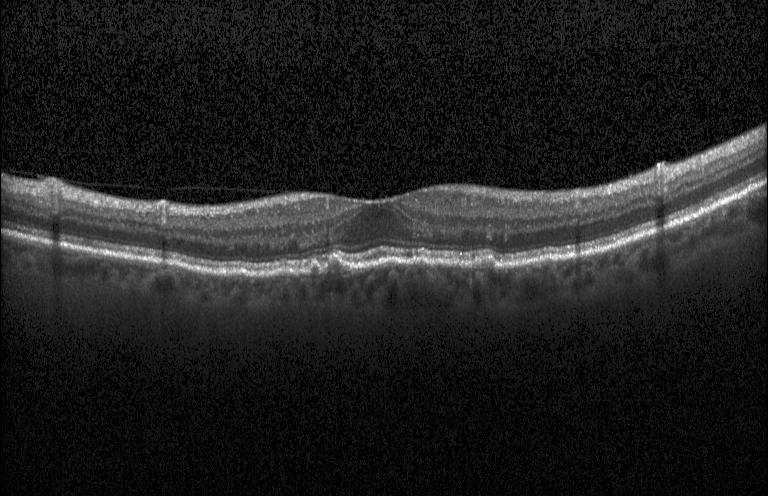 Macular OCT: multiple drusen.